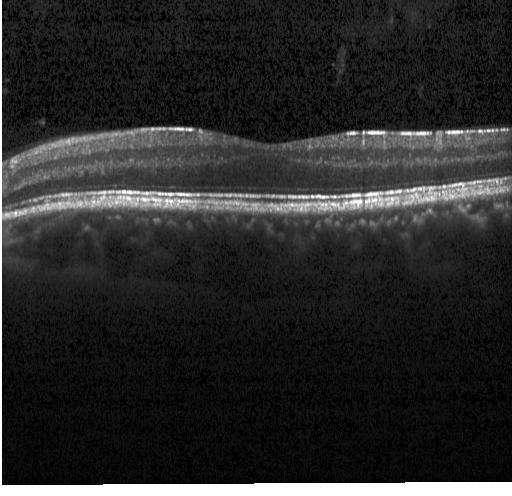

Retinal OCT B-scan
Diagnosis: no choroidal neovascularization, no diabetic macular edema, and no drusen.